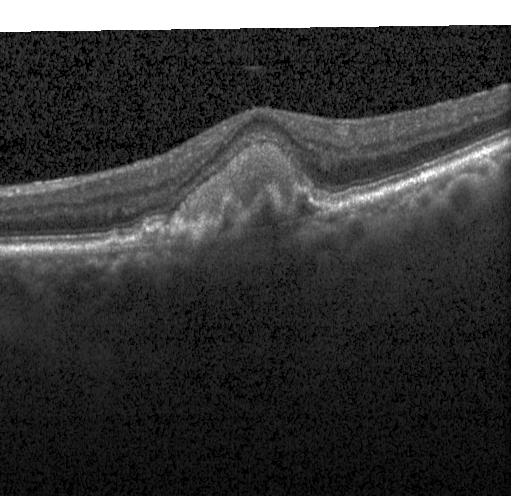

Centered on the fovea, optical coherence tomography scan
Finding: choroidal neovascularization.